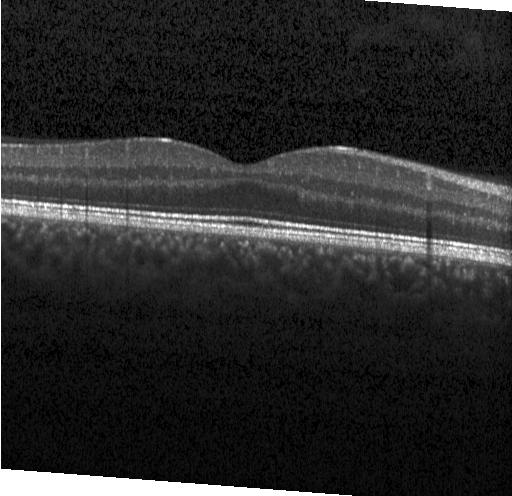
Optical coherence tomography scan.
The scan shows no CNV, no DME, and no drusen.